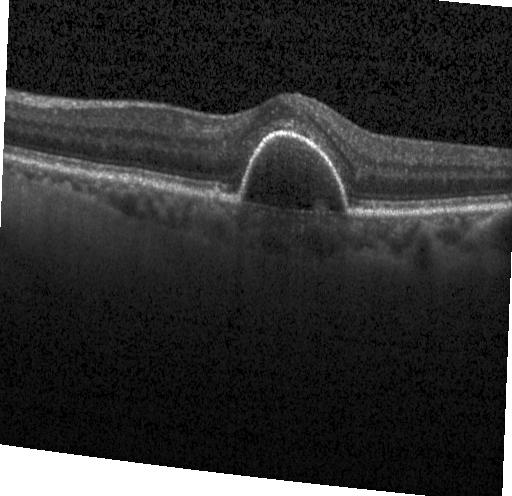 Macular scan · spectral-domain OCT · OCT line scan. Macular OCT: choroidal neovascularization.